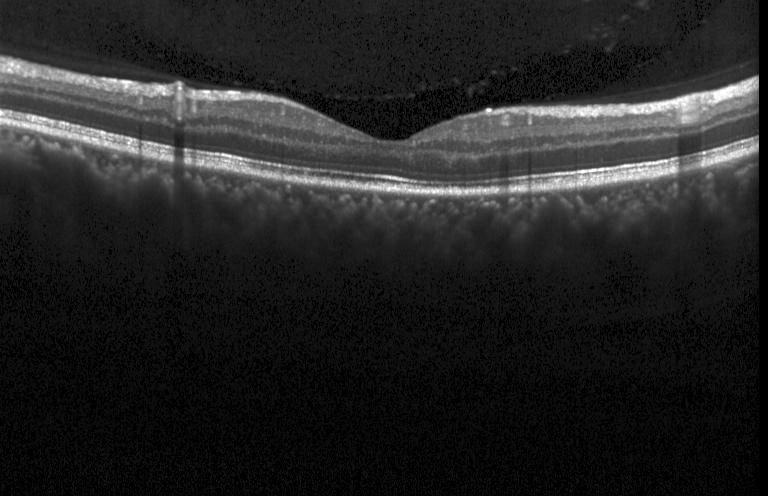 OCT B-scan. Diagnosis: no choroidal neovascularization, diabetic macular edema, or drusen.